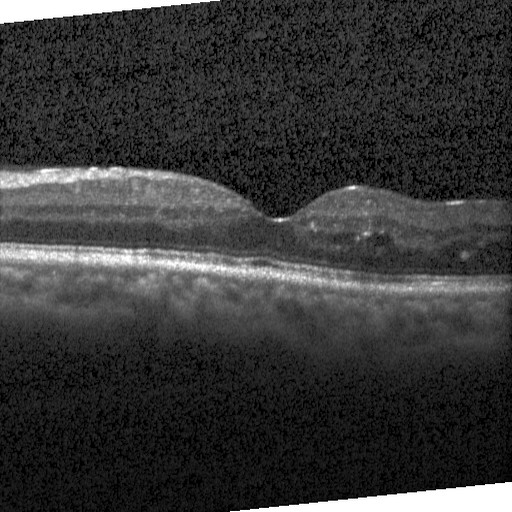
Horizontal scan through the fovea · retinal OCT cross-section · acquired on a Heidelberg Spectralis.
Impression: diabetic macular edema (DME).